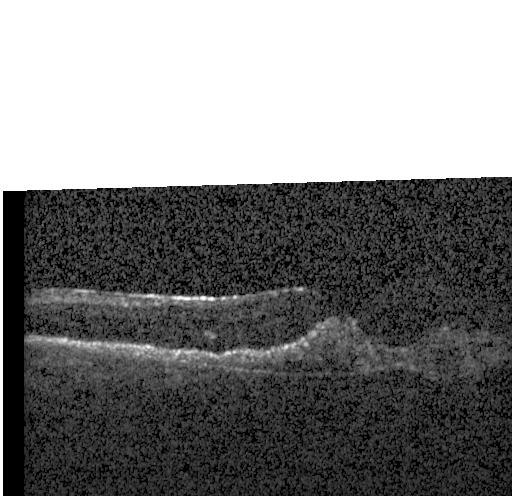 Diagnosis: choroidal neovascularization (CNV).